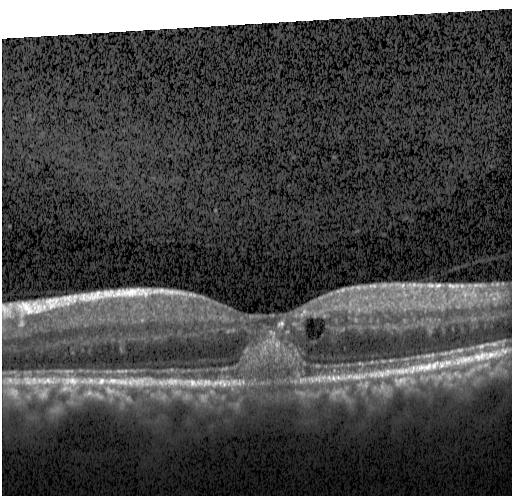 Centered on the fovea. Spectral-domain optical coherence tomography. Optical coherence tomography B-scan. Heidelberg Spectralis OCT system
Diagnosis: choroidal neovascularization (CNV).